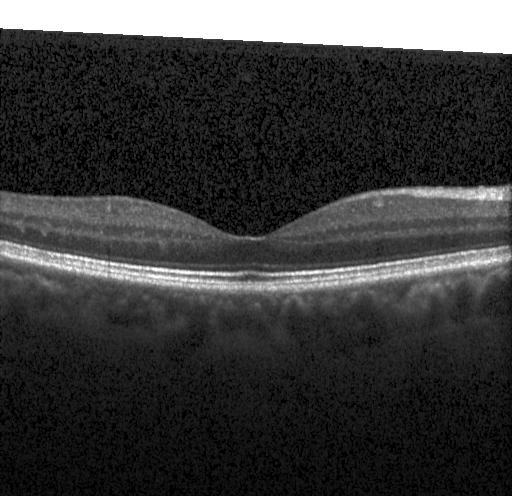

Macular scan, retinal OCT B-scan. Diagnosis: no choroidal neovascularization, no diabetic macular edema, and no drusen.